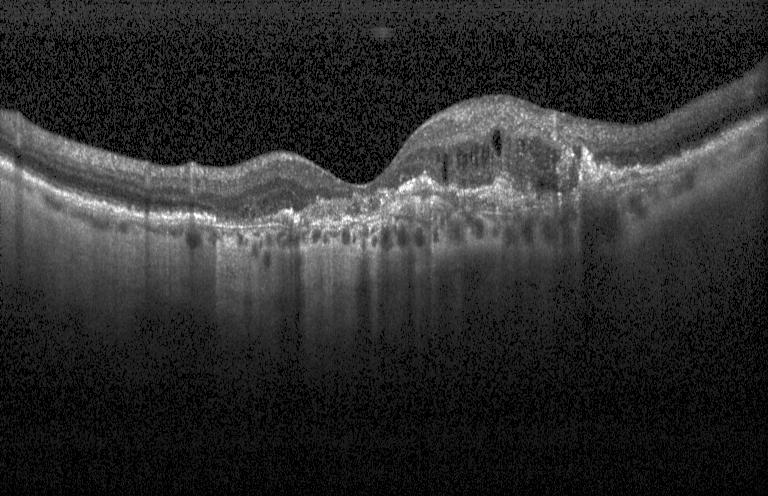

Retinal OCT B-scan
Finding: a choroidal neovascular membrane.